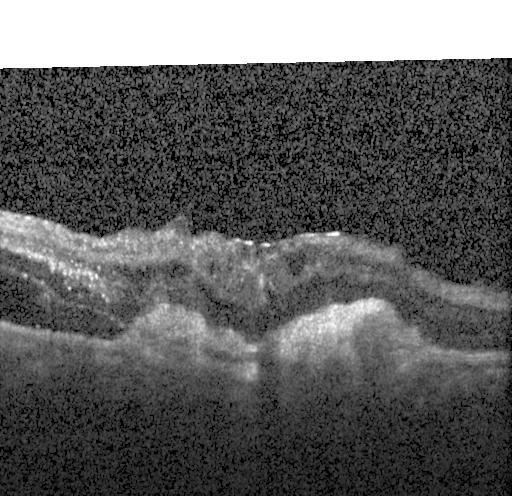

Acquired on a Heidelberg Spectralis · optical coherence tomography B-scan · spectral-domain optical coherence tomography · fovea-centered. This B-scan demonstrates choroidal neovascularization.